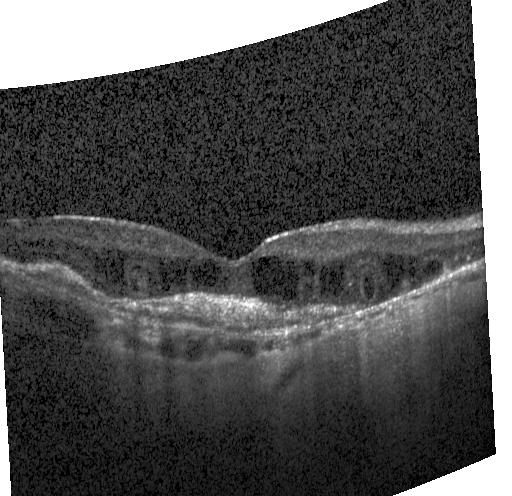 SD-OCT · through the macula · OCT line scan.
Choroidal neovascularization (CNV).